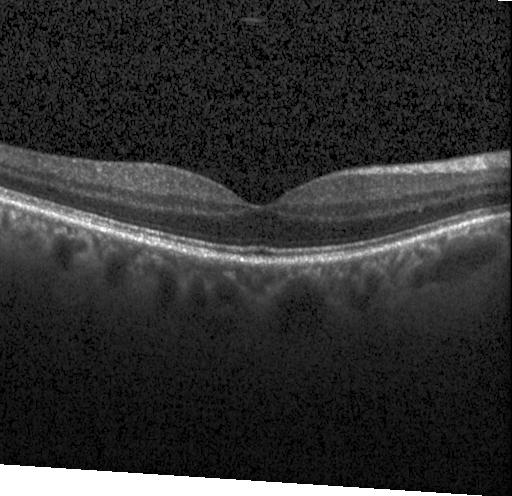
Finding: no CNV, DME, or drusen.